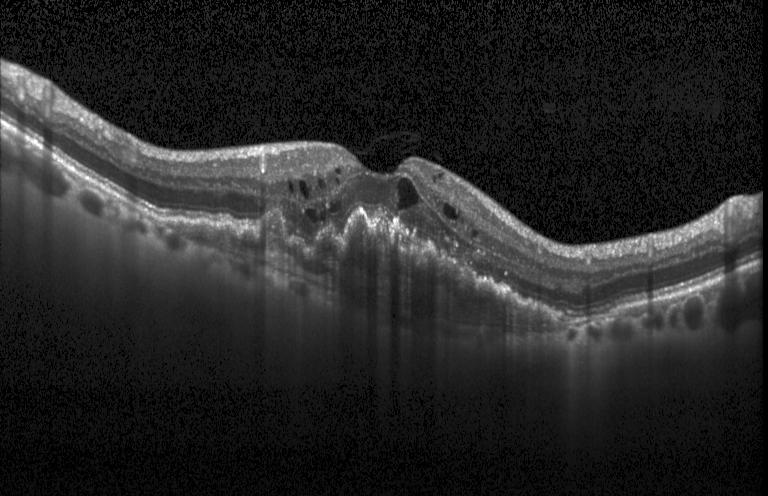
Finding: choroidal neovascularization.